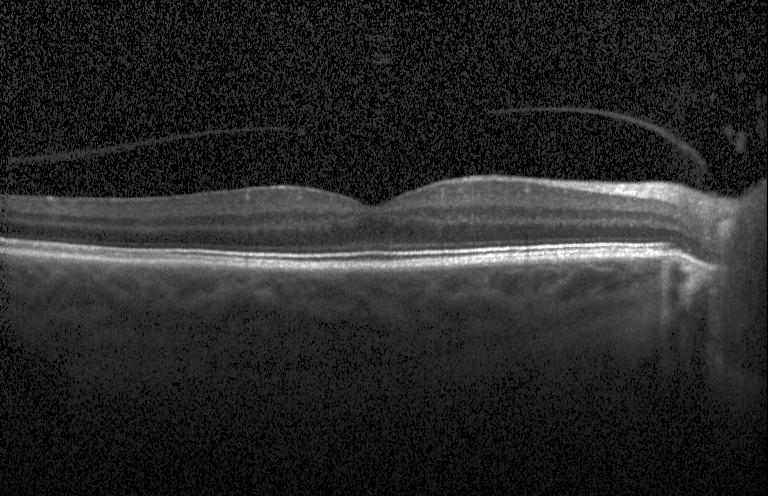 Retinal OCT B-scan · centered on the fovea · spectral-domain OCT.
The scan shows no CNV, no DME, and no drusen.